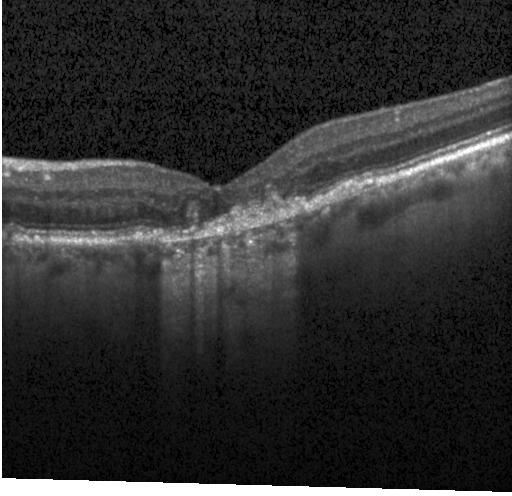

Optical coherence tomography scan. SD-OCT — This B-scan demonstrates choroidal neovascularization (CNV).